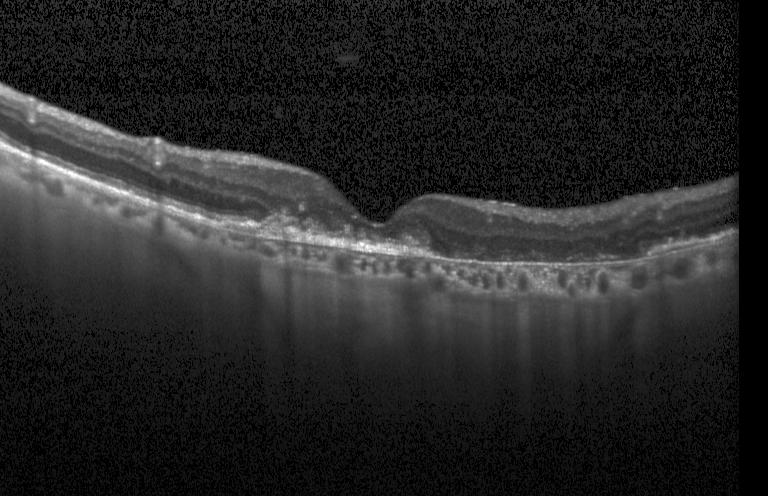 OCT B-scan; instrument: Heidelberg Spectralis; spectral-domain OCT.
This B-scan demonstrates choroidal neovascularization (CNV).